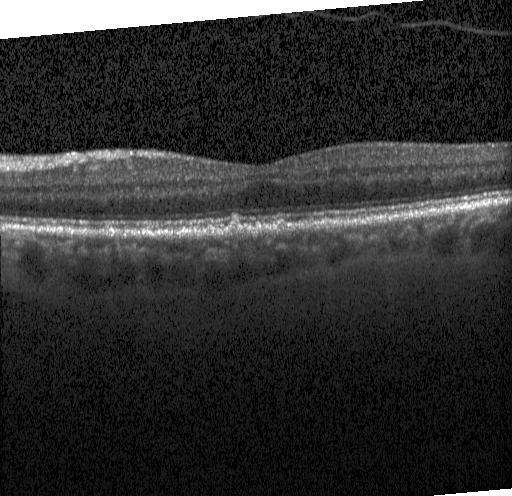

Macular OCT demonstrating drusen.